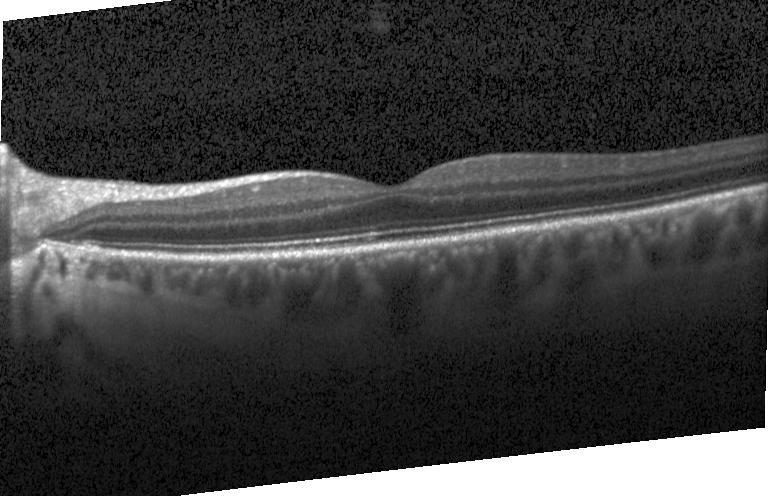

Macular OCT demonstrating no choroidal neovascularization, no diabetic macular edema, and no drusen.